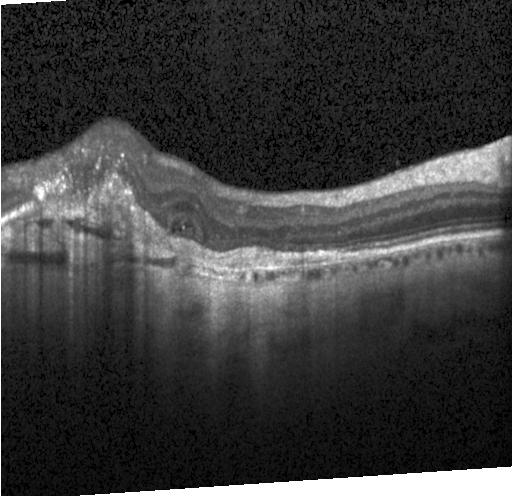 OCT line scan, Heidelberg Spectralis OCT system.
OCT finding: a choroidal neovascular membrane.